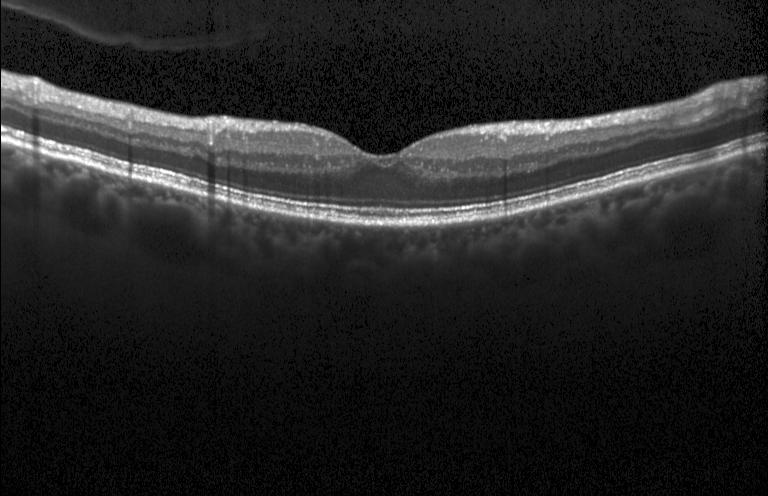
Retinal OCT cross-section showing no CNV, no DME, and no drusen.